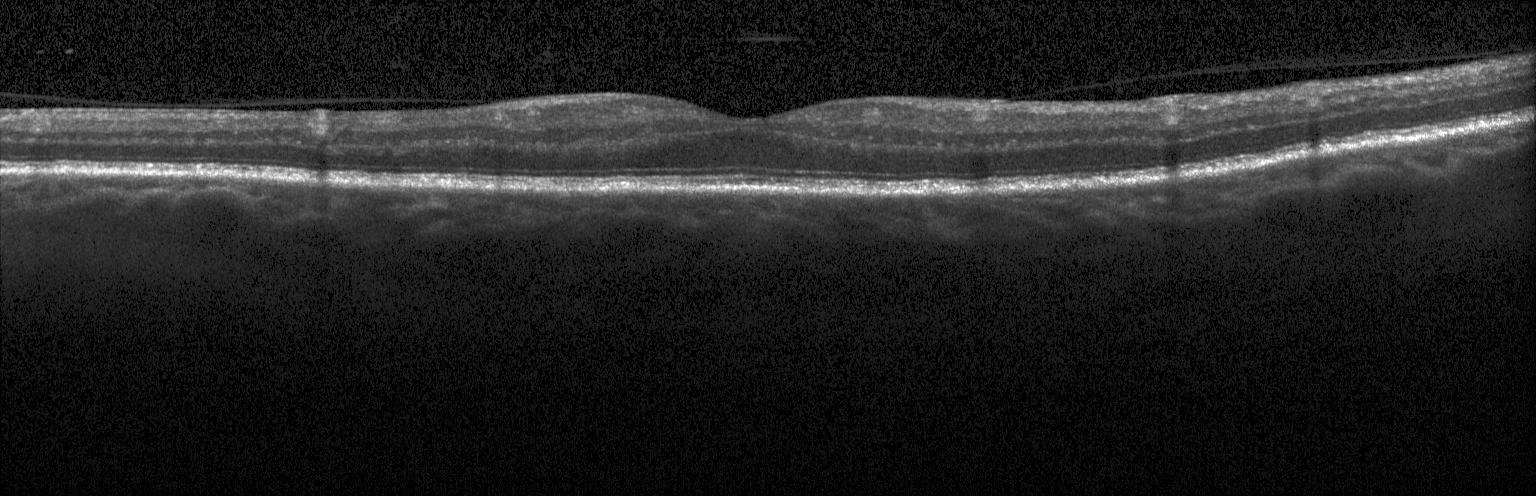
Horizontal scan through the fovea. OCT B-scan — Dx: no choroidal neovascularization, diabetic macular edema, or drusen.